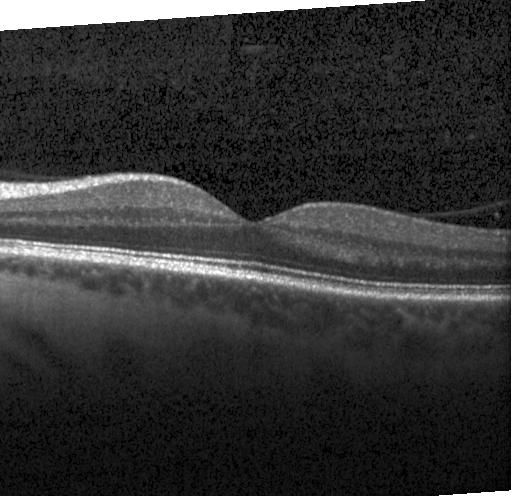 Diagnosis: no evidence of CNV, DME, or drusen.